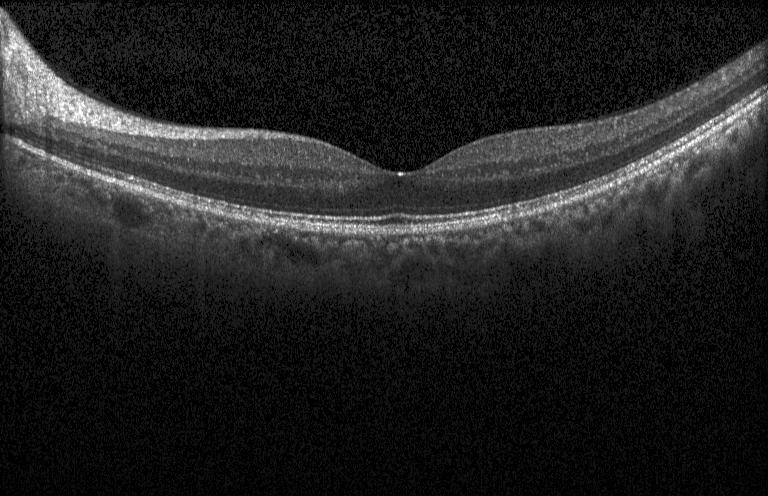

Retinal OCT B-scan — This B-scan demonstrates no choroidal neovascularization, diabetic macular edema, or drusen.